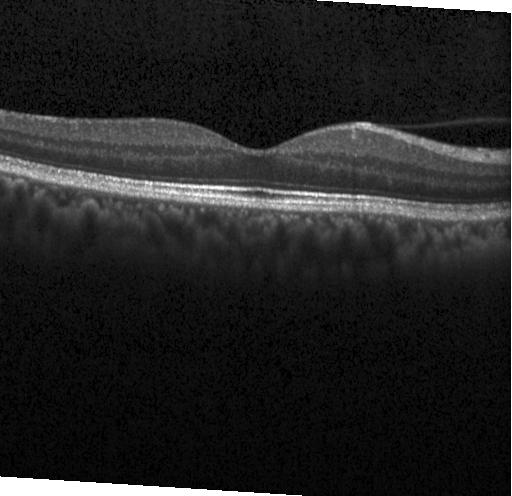

Spectral-domain OCT B-scan: neither choroidal neovascularization, diabetic macular edema, nor drusen.